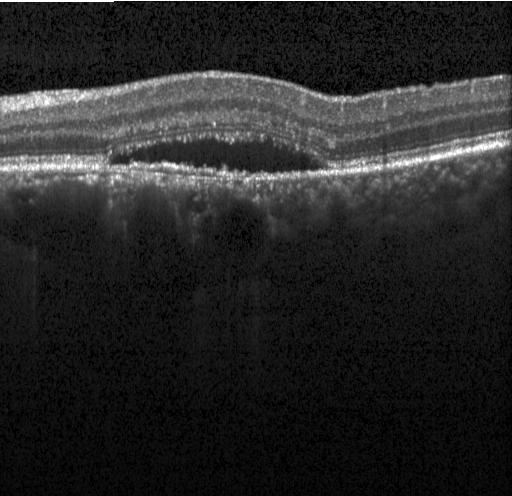 Retinal OCT cross-section, SD-OCT, horizontal scan through the fovea, acquired on a Heidelberg Spectralis.
Assessment: a choroidal neovascular membrane.